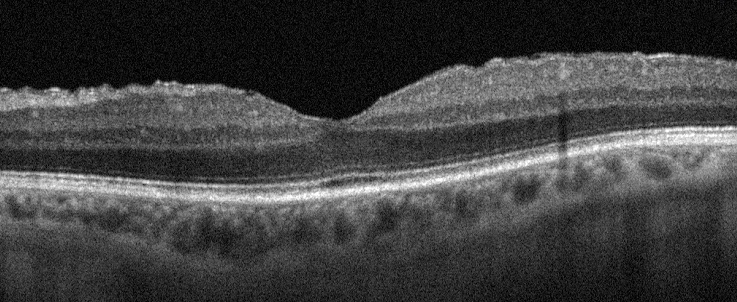

Acquired on an Optovue Avanti RTVue XR. OCT line scan. Fovea-centered — Impression: ERM.